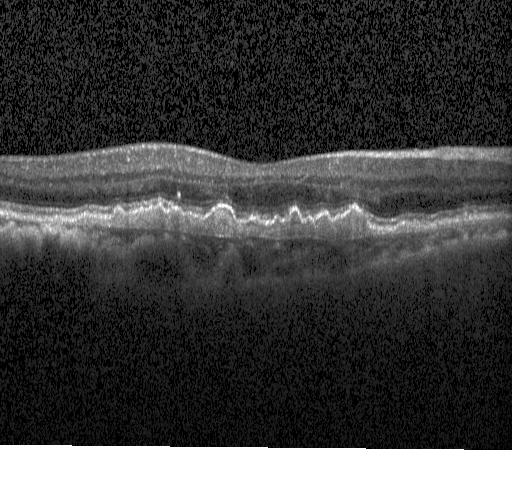

Optical coherence tomography scan. Finding: CNV.